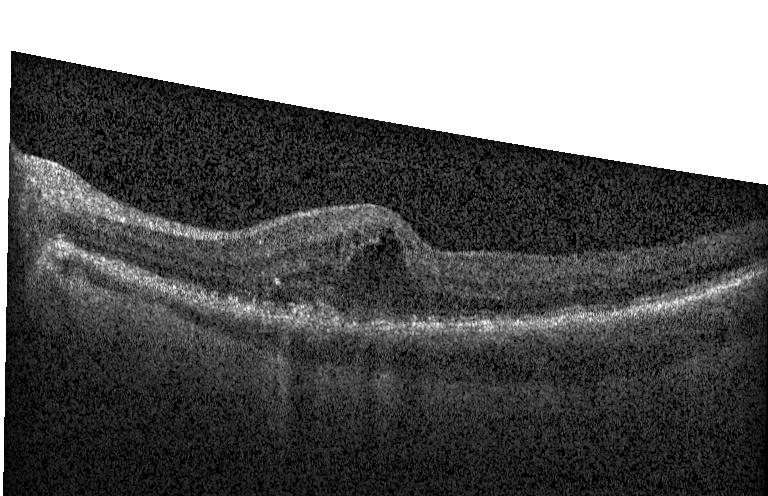
Impression: a choroidal neovascular membrane.